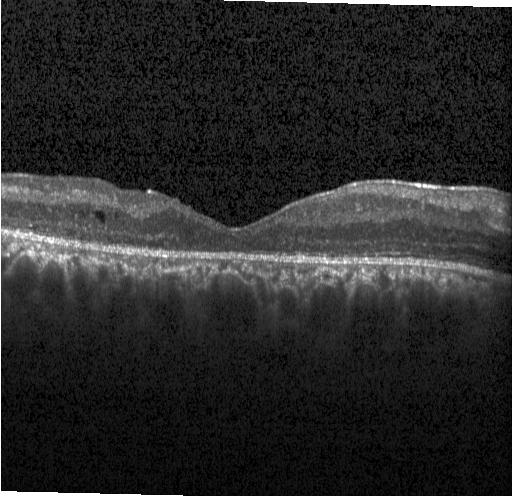

Finding: diabetic macular edema (DME).